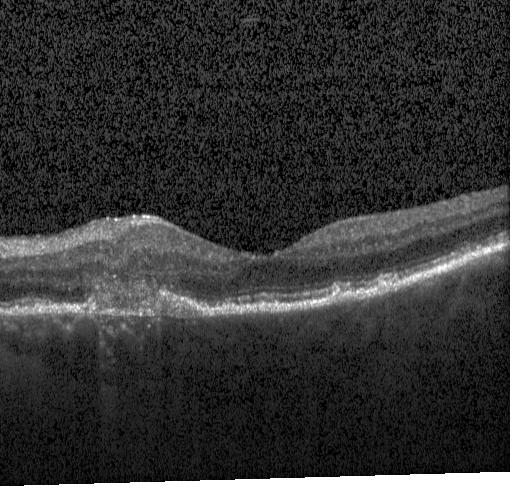
OCT line scan. SD-OCT. Fovea-centered. Dx: a choroidal neovascular membrane.